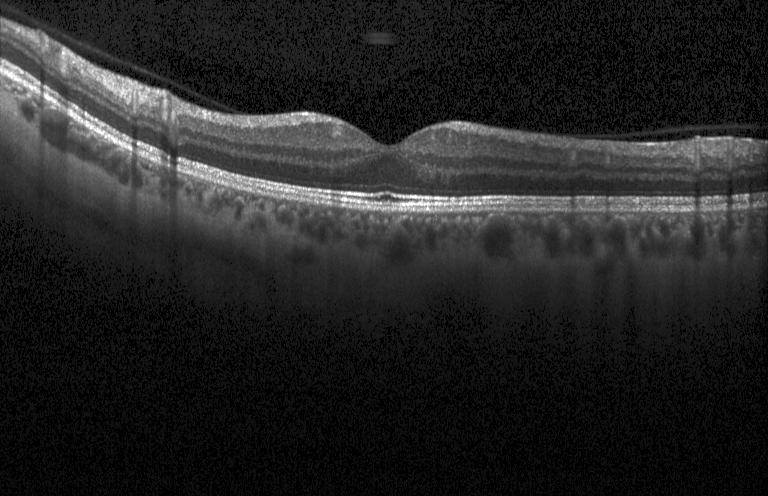 Retinal OCT cross-section showing no evidence of CNV, DME, or drusen.